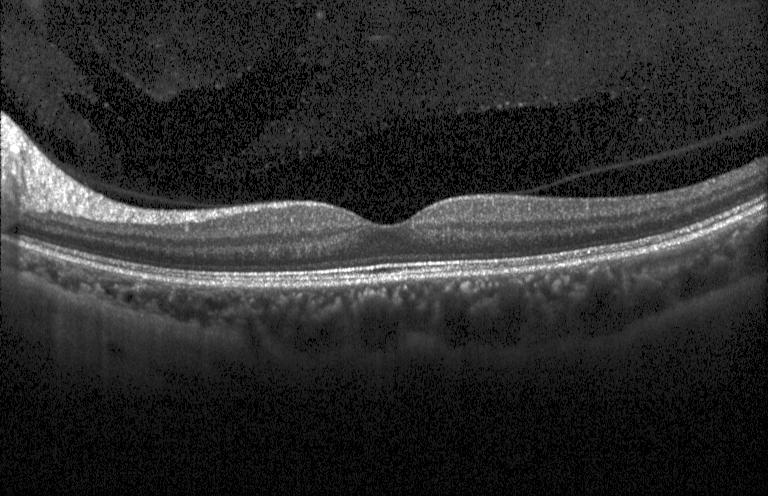 Finding: no choroidal neovascularization, diabetic macular edema, or drusen.